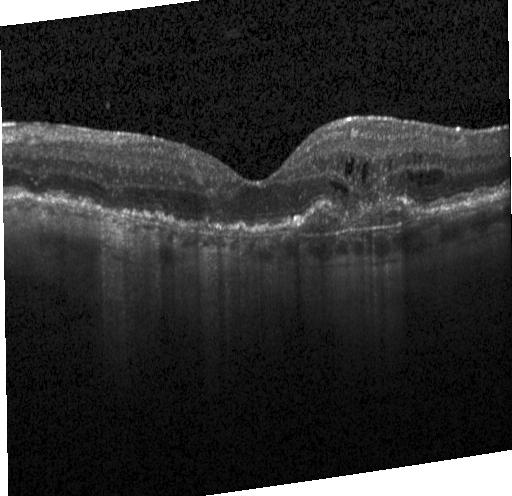

SD-OCT. Centered on the fovea. Optical coherence tomography scan — Dx: choroidal neovascularization (CNV).